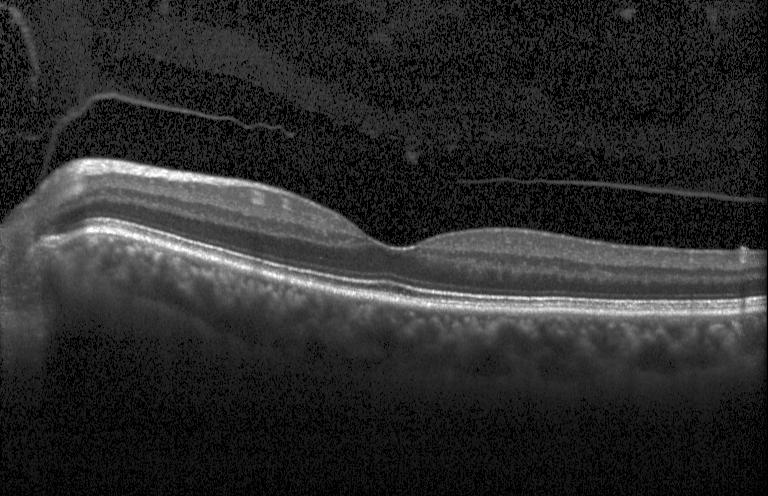
OCT scan showing neither choroidal neovascularization, diabetic macular edema, nor drusen.